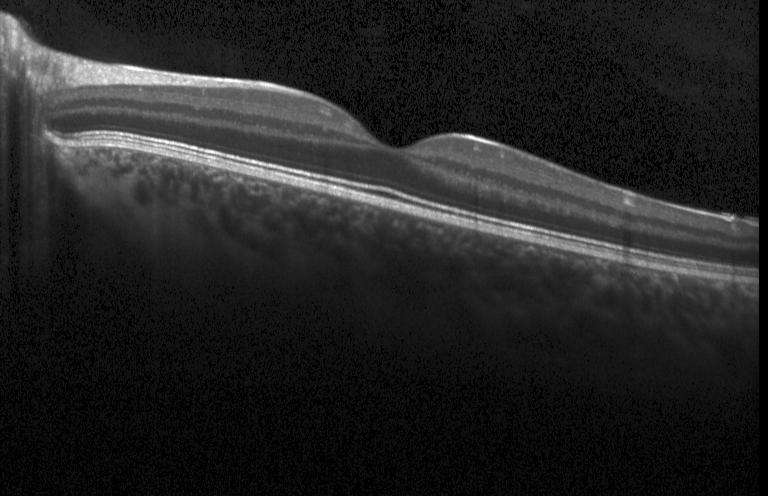

Optical coherence tomography scan.
This B-scan demonstrates no CNV, no DME, and no drusen.